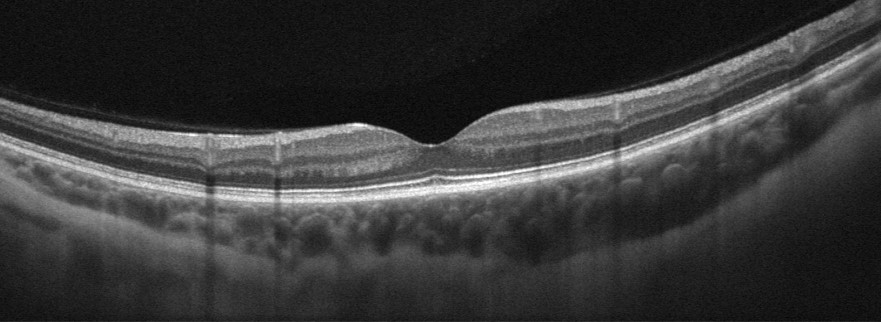 Impression: absence of AMD, DME, ERM, RAO, RVO, and vitreomacular interface disease.